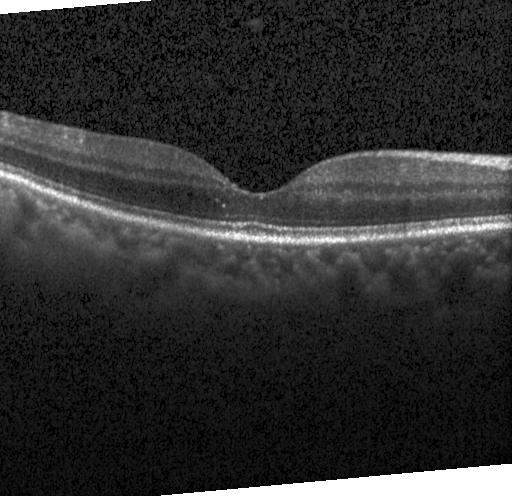
OCT B-scan · spectral-domain optical coherence tomography. Diagnosis: no CNV, no DME, and no drusen.